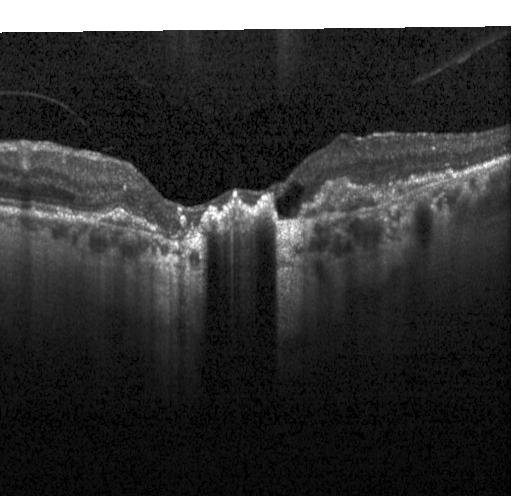 Finding: choroidal neovascularization.